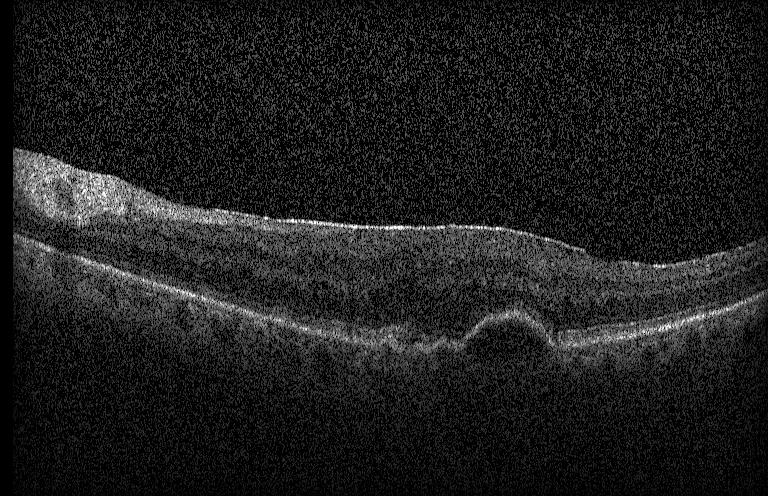 Impression: choroidal neovascularization (CNV).